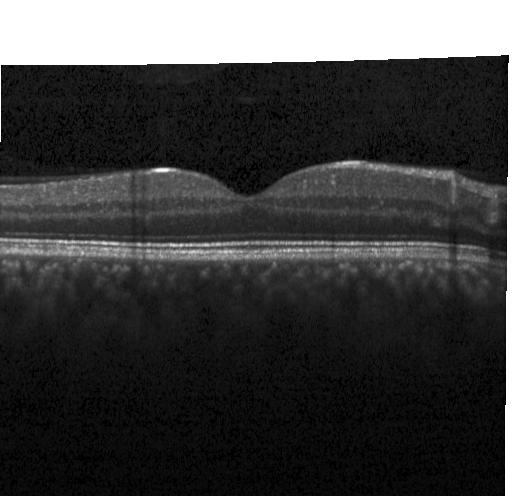

Finding: no choroidal neovascularization, no diabetic macular edema, and no drusen.